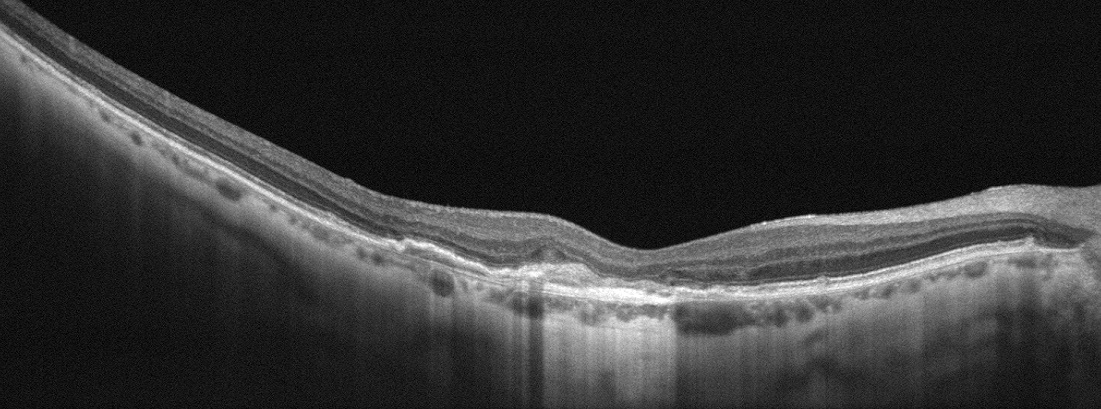
Instrument: Optovue Avanti RTVue XR · retinal OCT B-scan · macular scan
Diagnosis: AMD.